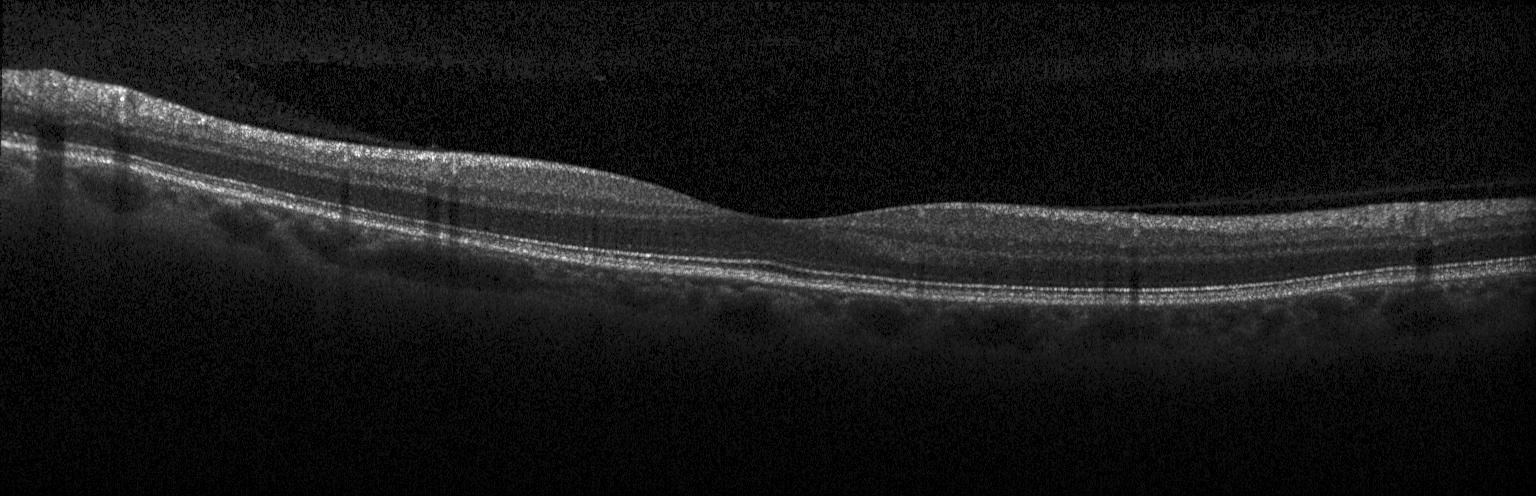

Optical coherence tomography B-scan.
Diagnosis: no choroidal neovascularization, diabetic macular edema, or drusen.